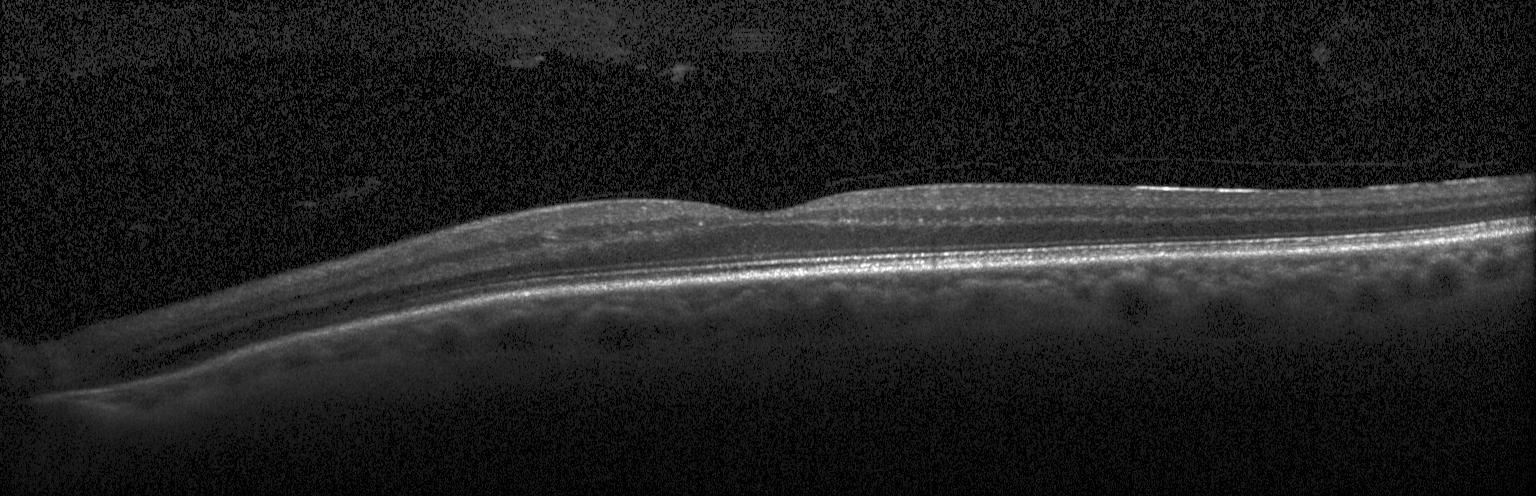 Optical coherence tomography scan. Spectral-domain optical coherence tomography. Acquired on a Heidelberg Spectralis. Diagnosis: no choroidal neovascularization, no diabetic macular edema, and no drusen.